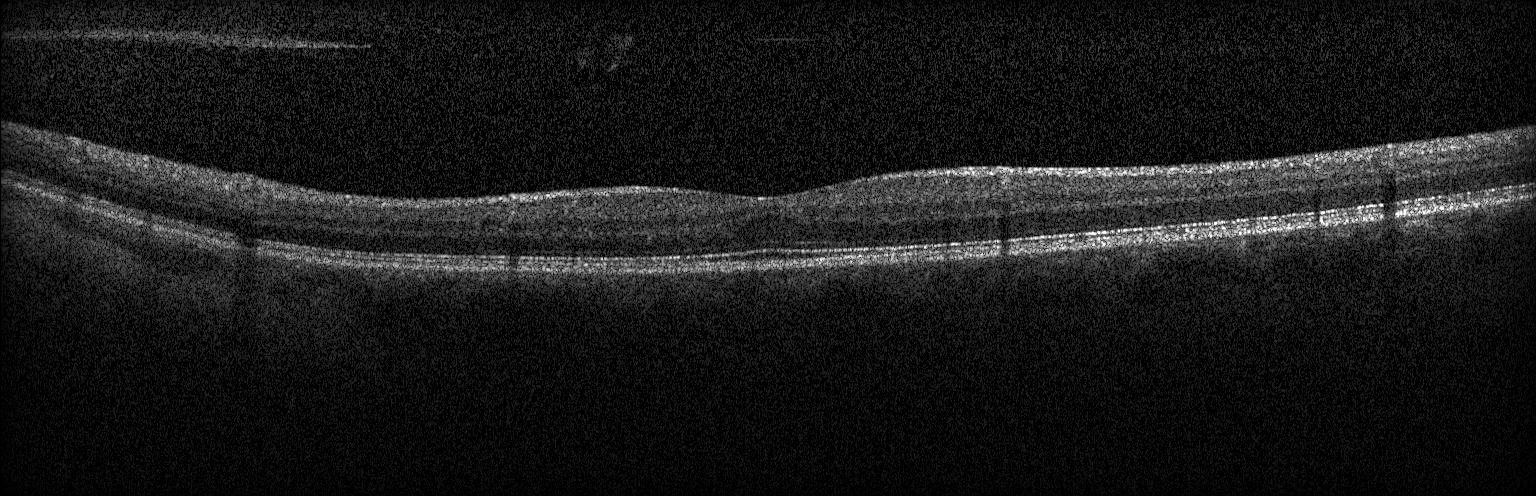

Spectral-domain OCT B-scan: no evidence of CNV, DME, or drusen.